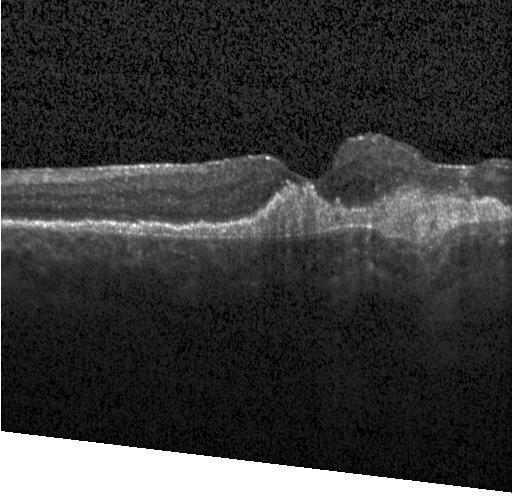 Assessment: a choroidal neovascular membrane.